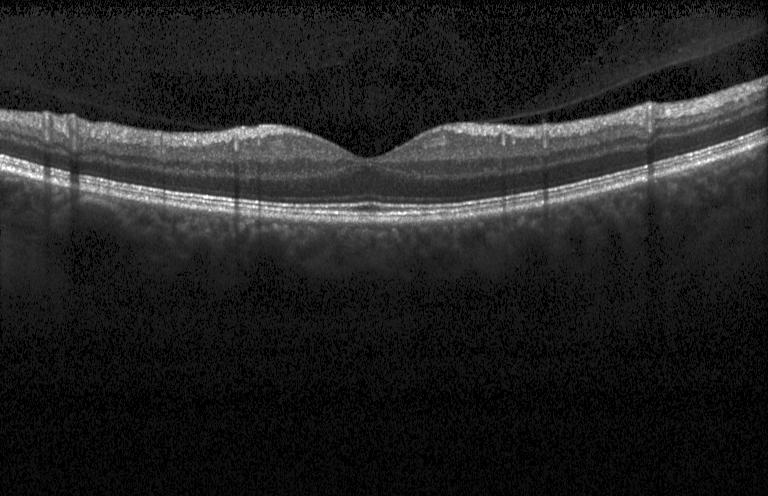

Retinal OCT cross-section · Heidelberg Spectralis OCT system · through the macula.
Finding: no CNV, no DME, and no drusen.